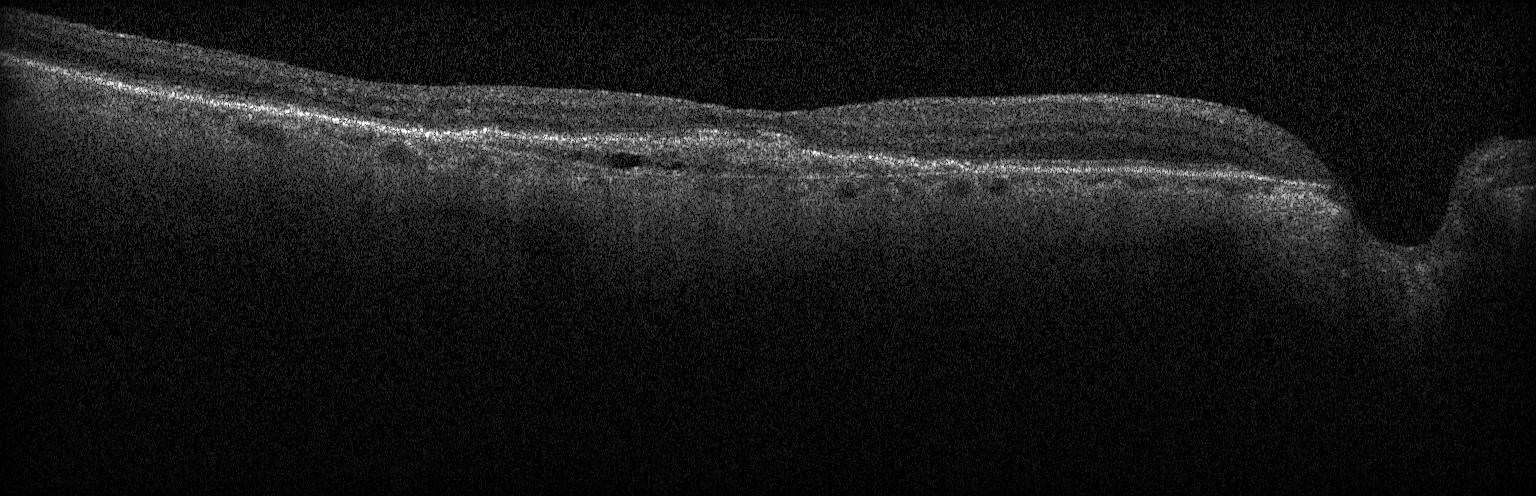
Retinal OCT cross-section — Impression: choroidal neovascularization (CNV).